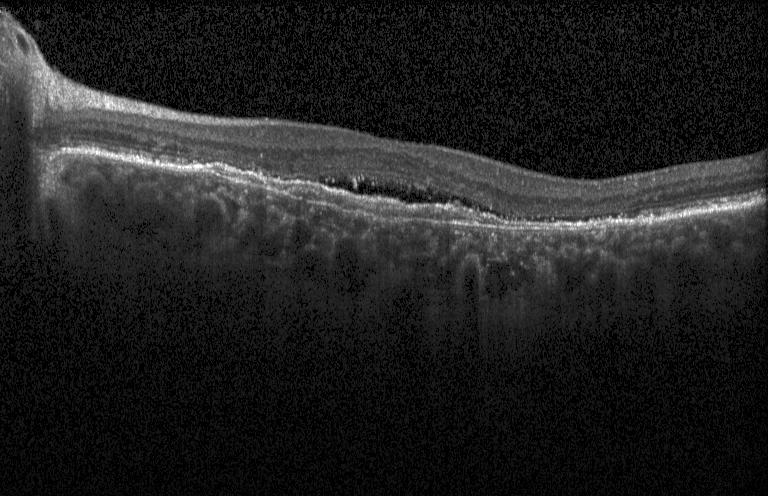
Impression: a choroidal neovascular membrane.